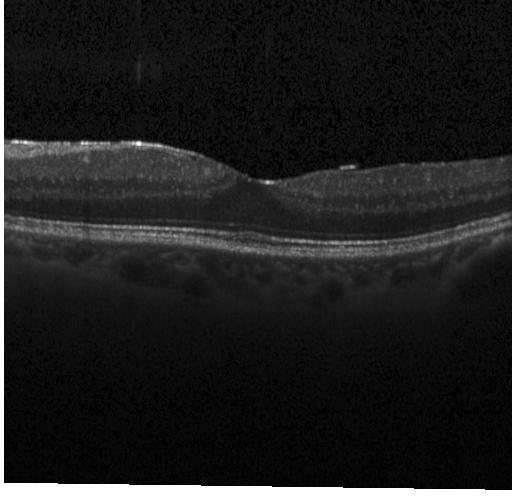

OCT finding: no CNV, DME, or drusen.